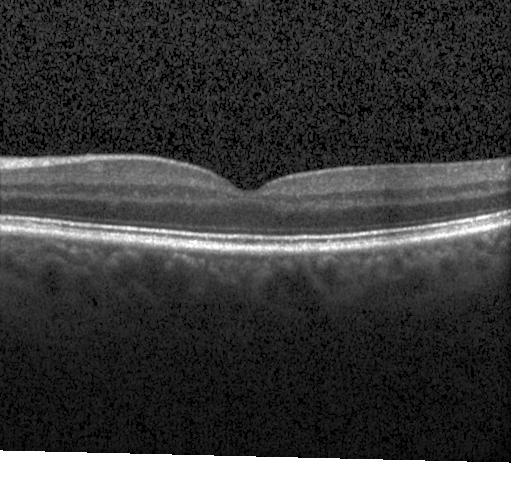 Macular scan. Spectral-domain optical coherence tomography. OCT line scan. OCT finding: no CNV, DME, or drusen.